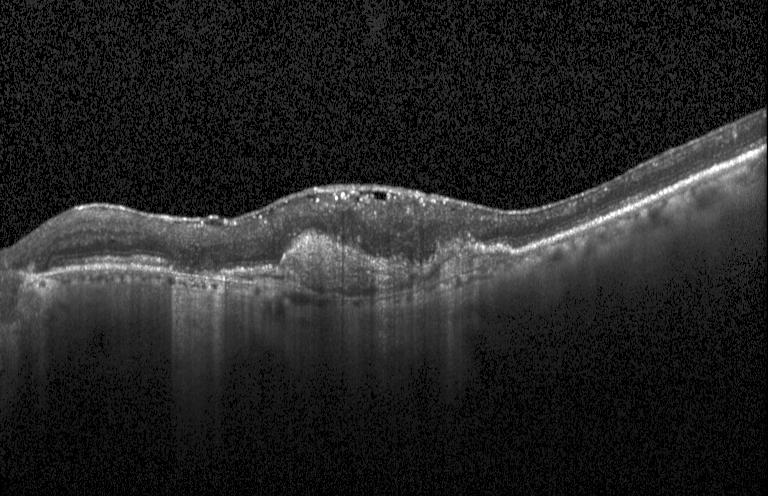

Retinal OCT cross-section.
Diagnosis: CNV.